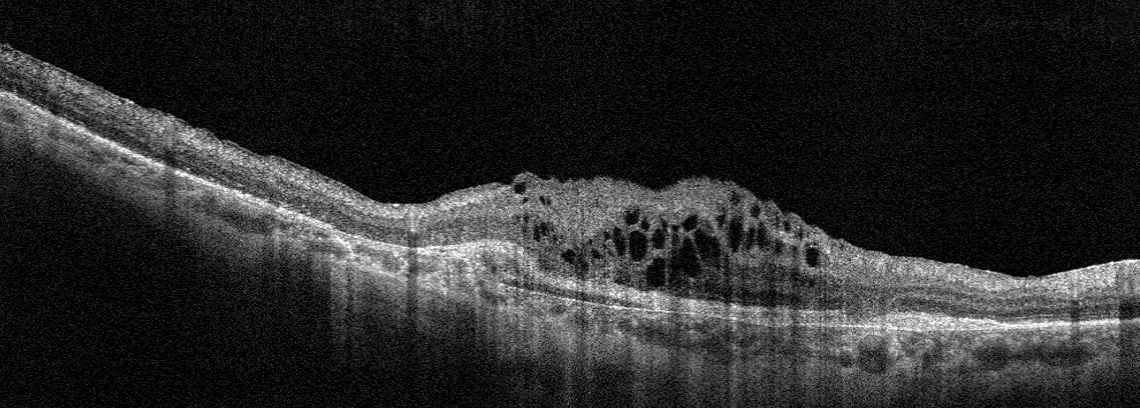

AMD.